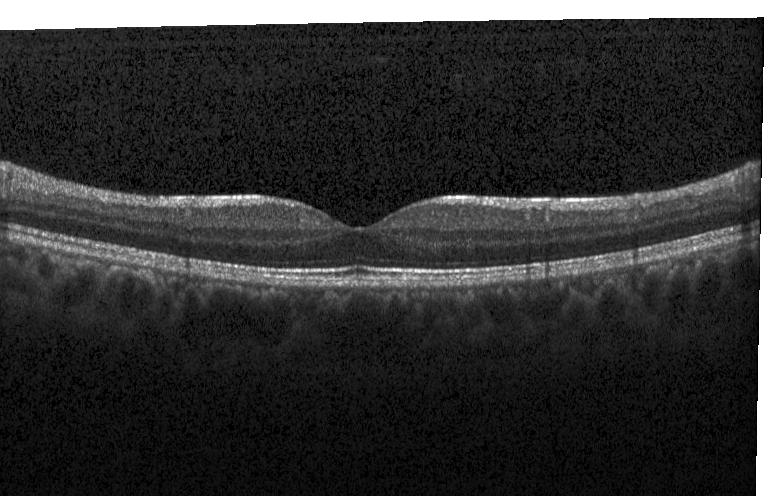

OCT B-scan — Assessment: neither CNV, DME, nor drusen.